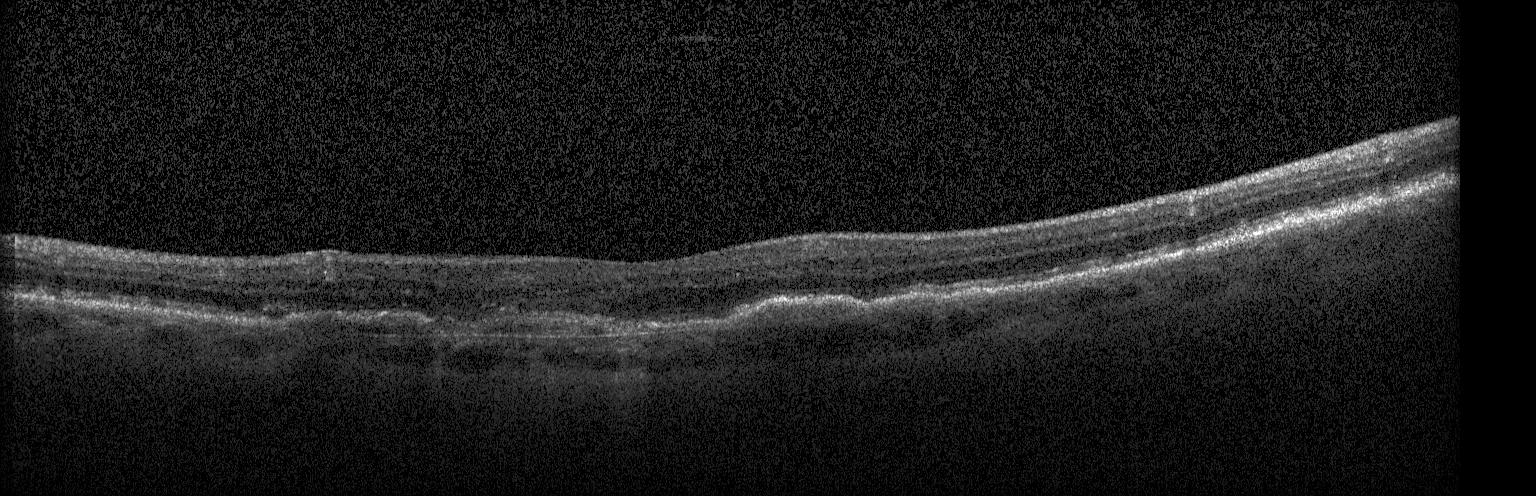
Acquired on a Heidelberg Spectralis · SD-OCT · optical coherence tomography scan · macular scan.
The scan shows choroidal neovascularization (CNV).